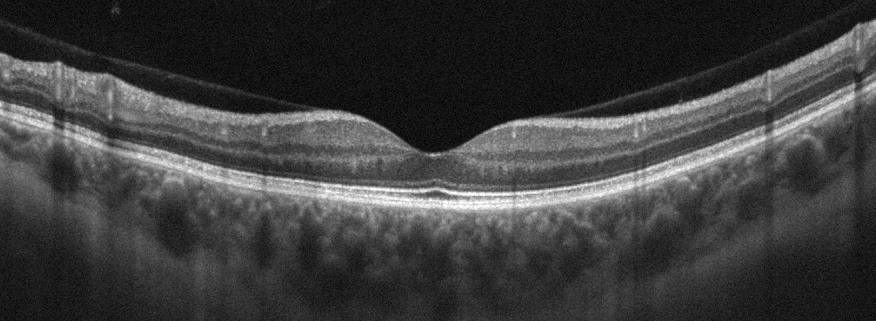 Optovue Avanti RTVue XR; OCT B-scan. Finding: absence of AMD, DME, ERM, RAO, RVO, and vitreomacular interface disease.